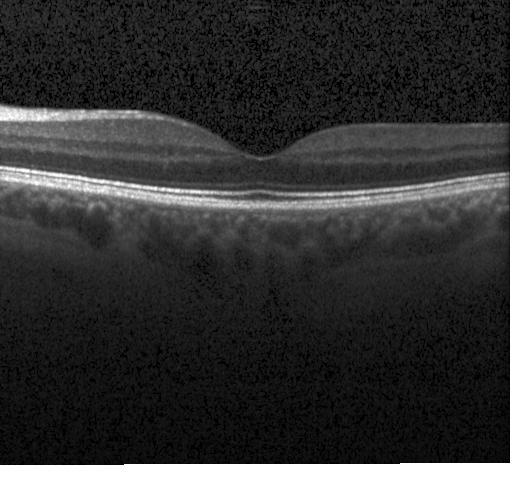

Heidelberg Spectralis OCT system. Centered on the fovea. Spectral-domain optical coherence tomography. OCT B-scan.
The scan shows neither choroidal neovascularization, diabetic macular edema, nor drusen.